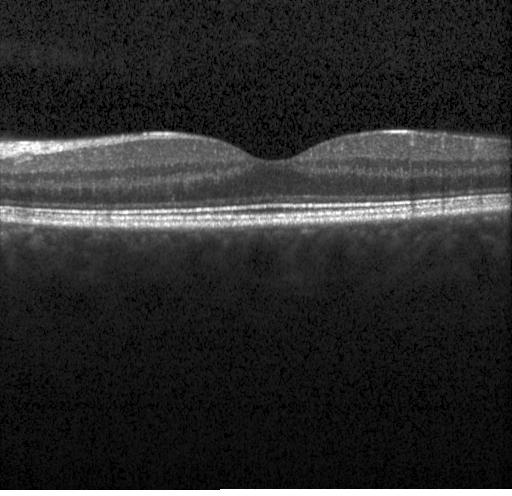
Spectral-domain optical coherence tomography · retinal OCT cross-section · Heidelberg Spectralis OCT system · fovea-centered
This B-scan demonstrates no evidence of CNV, DME, or drusen.